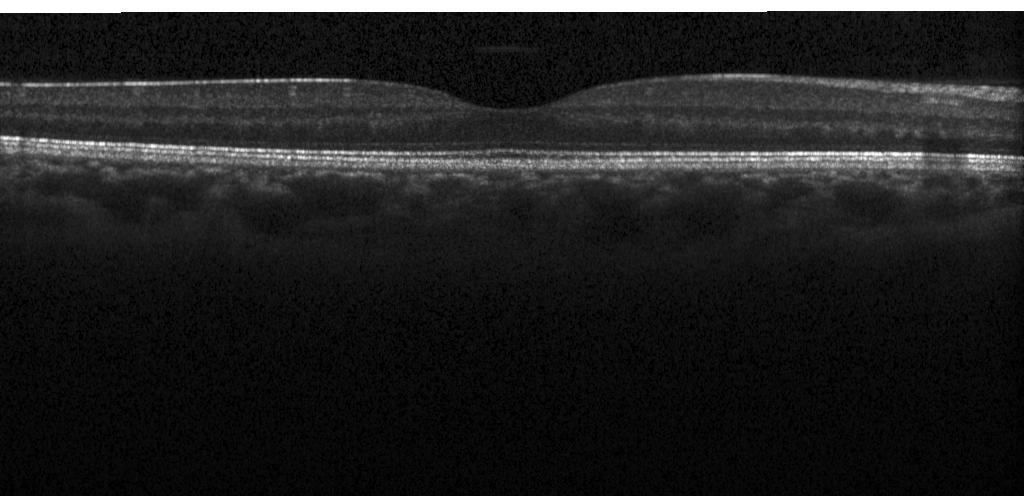

OCT finding: no CNV, no DME, and no drusen.